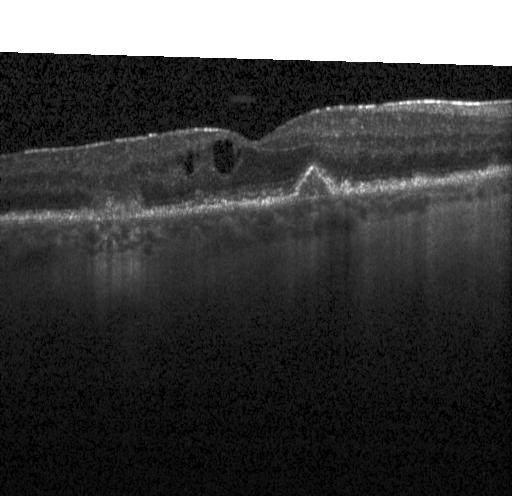 Fovea-centered, spectral-domain optical coherence tomography, retinal OCT B-scan
Finding: diabetic macular edema (DME).